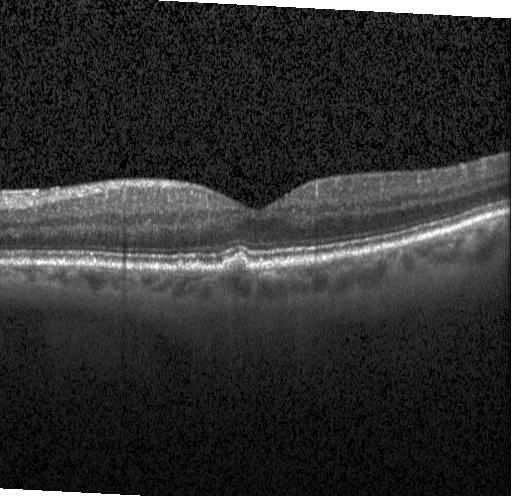
OCT B-scan · macular scan.
Macular OCT: drusen.